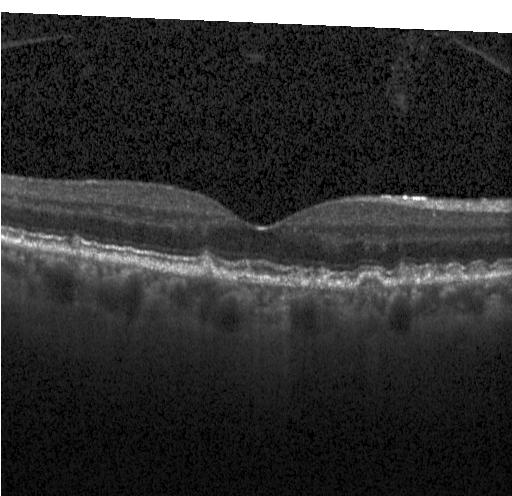

Retinal OCT B-scan.
Macular OCT: drusen.